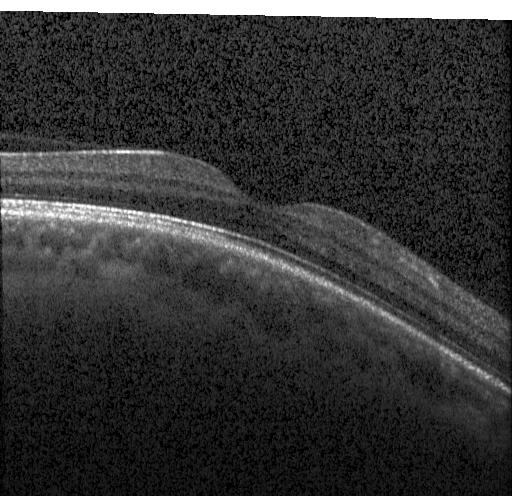

Optical coherence tomography scan.
No choroidal neovascularization, diabetic macular edema, or drusen.